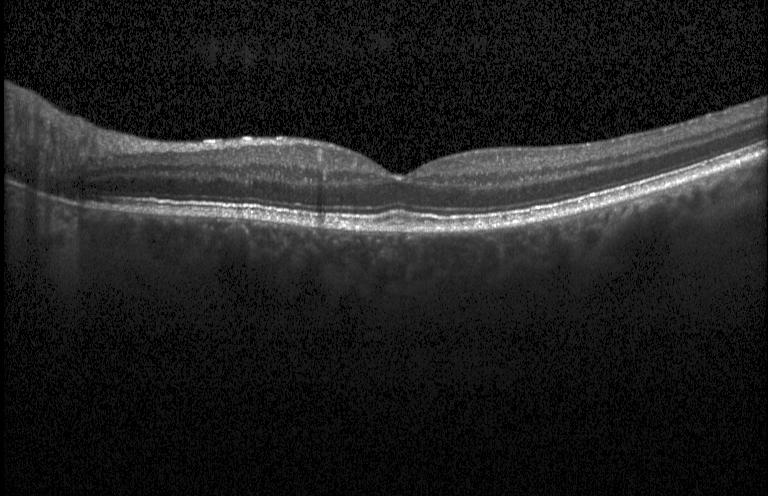

Optical coherence tomography scan
No choroidal neovascularization, no diabetic macular edema, and no drusen.